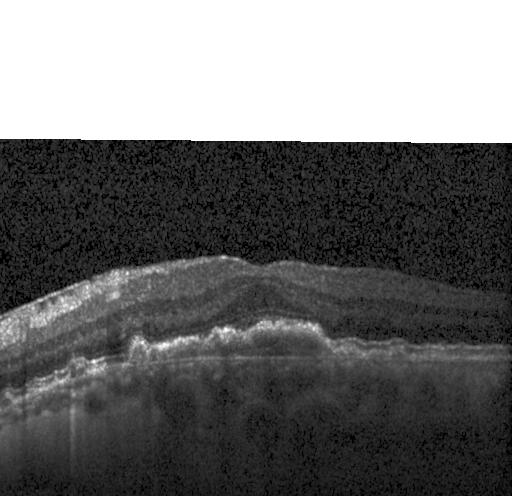

Heidelberg Spectralis OCT system, centered on the fovea, retinal OCT B-scan — OCT finding: a choroidal neovascular membrane.